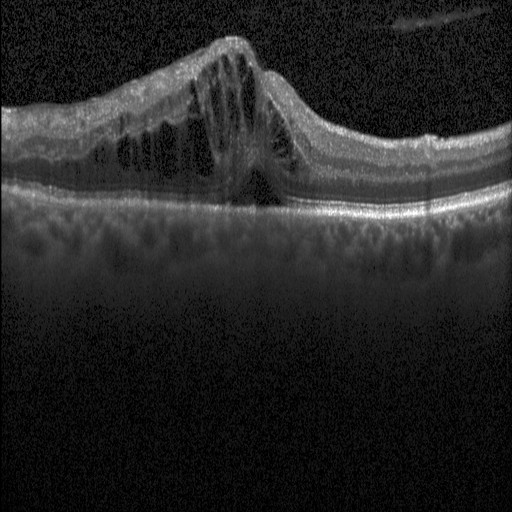 Optical coherence tomography scan. Spectral-domain OCT. Heidelberg Spectralis. Through the macula.
Assessment: diabetic macular edema.